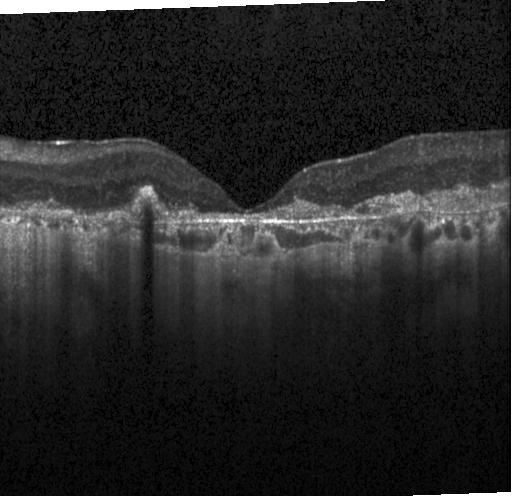 Retinal OCT cross-section. Heidelberg Spectralis — Diagnosis: choroidal neovascularization.